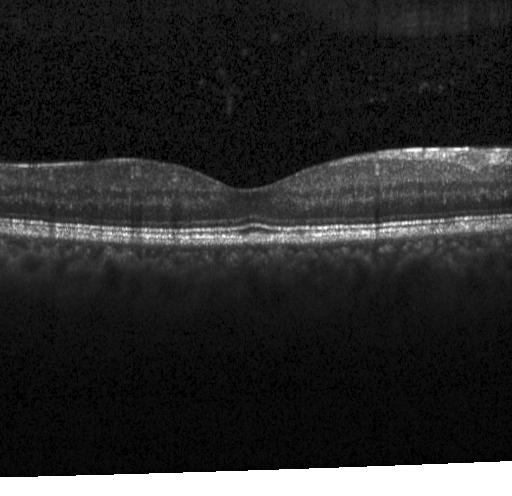
Fovea-centered. OCT B-scan. Instrument: Heidelberg Spectralis. Dx: no evidence of choroidal neovascularization, diabetic macular edema, or drusen.